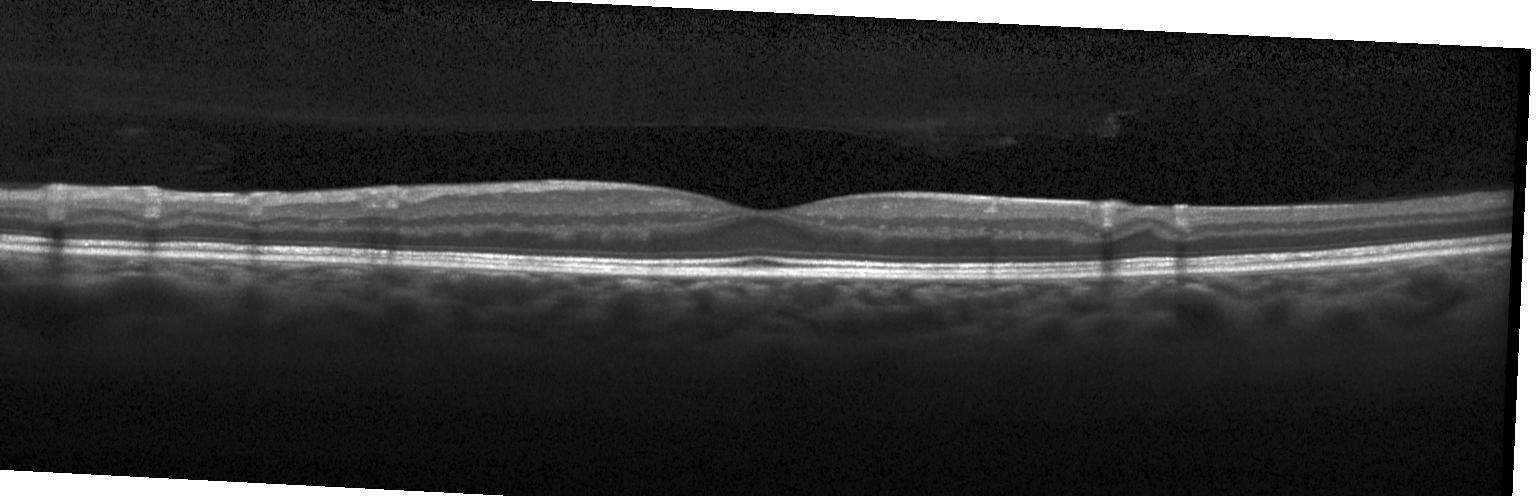

Retinal OCT cross-section — Diagnosis: no choroidal neovascularization, no diabetic macular edema, and no drusen.